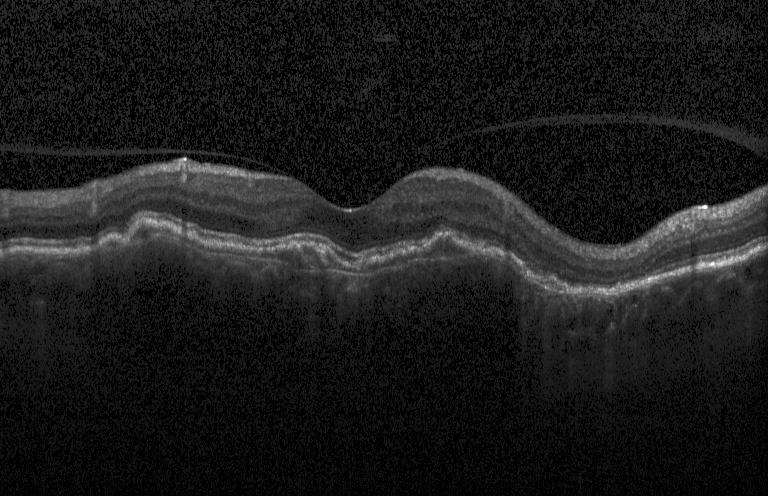 Retinal OCT cross-section showing choroidal neovascularization (CNV).